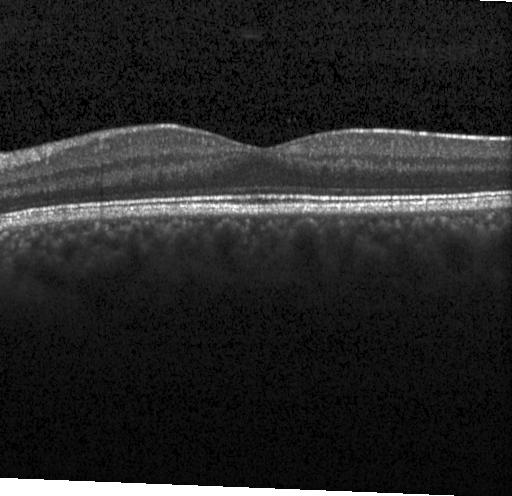
OCT line scan
No CNV, no DME, and no drusen.